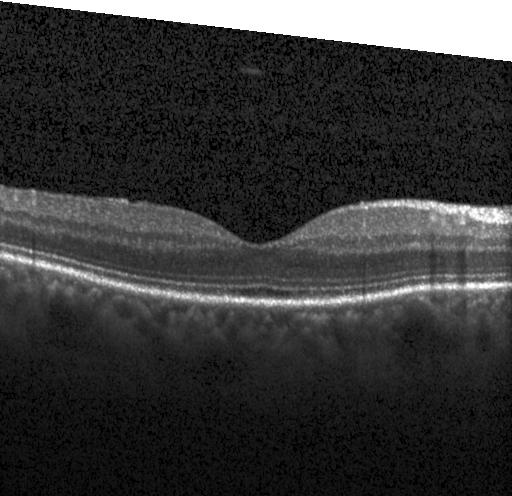

Optical coherence tomography scan. The scan shows no choroidal neovascularization, diabetic macular edema, or drusen.